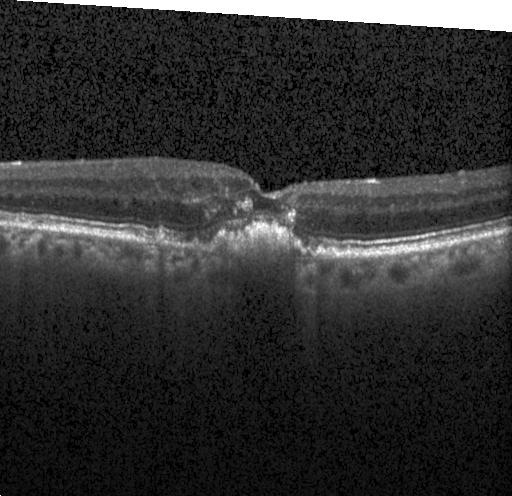
OCT B-scan
Diagnosis: choroidal neovascularization (CNV).